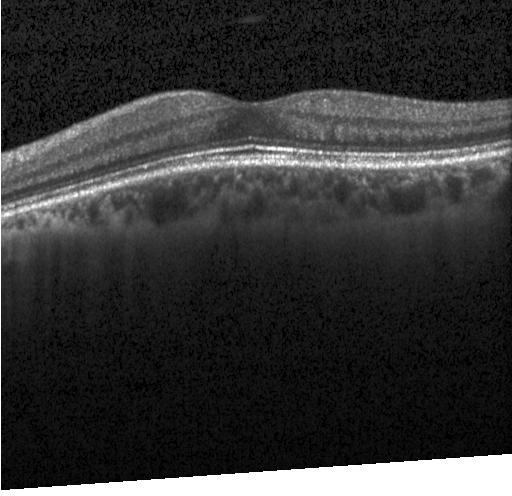 Dx: no evidence of choroidal neovascularization, diabetic macular edema, or drusen.